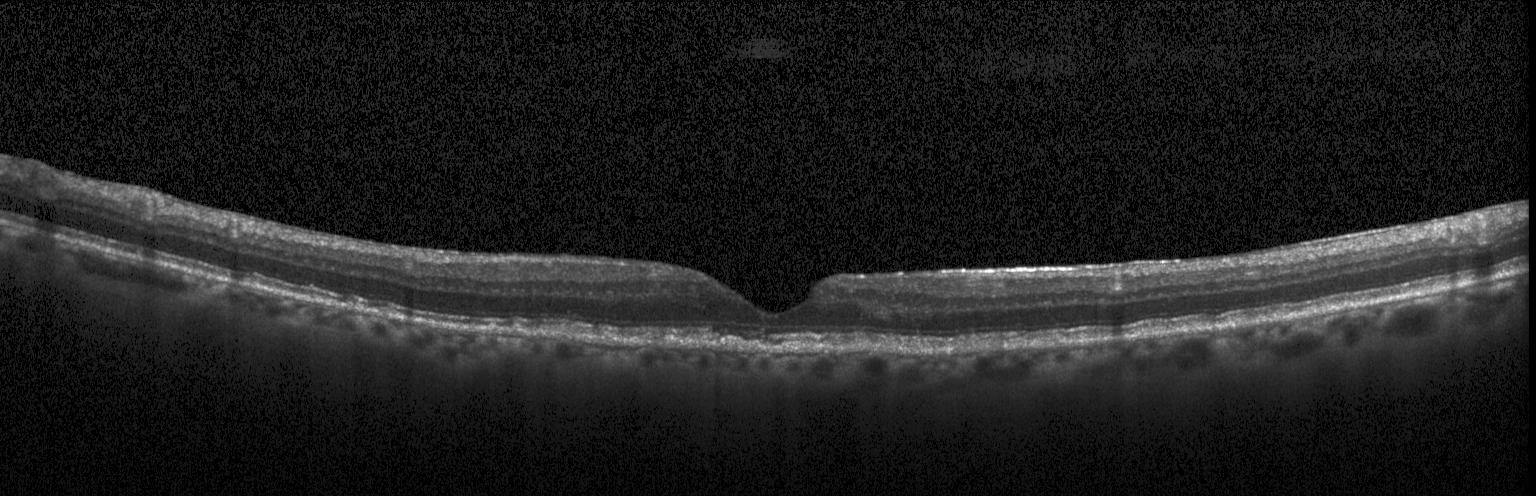

Optical coherence tomography scan, Heidelberg Spectralis.
Impression: multiple drusen.